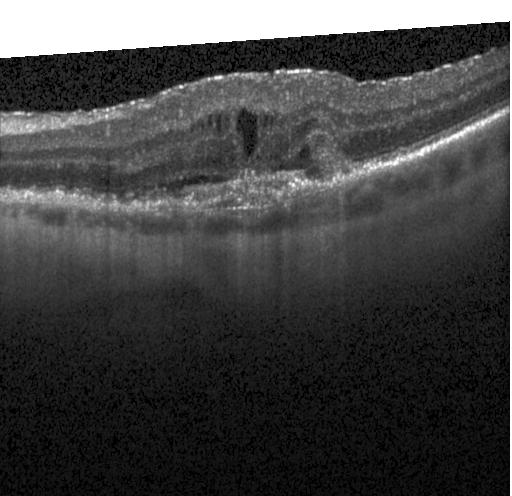 Impression: choroidal neovascularization (CNV).